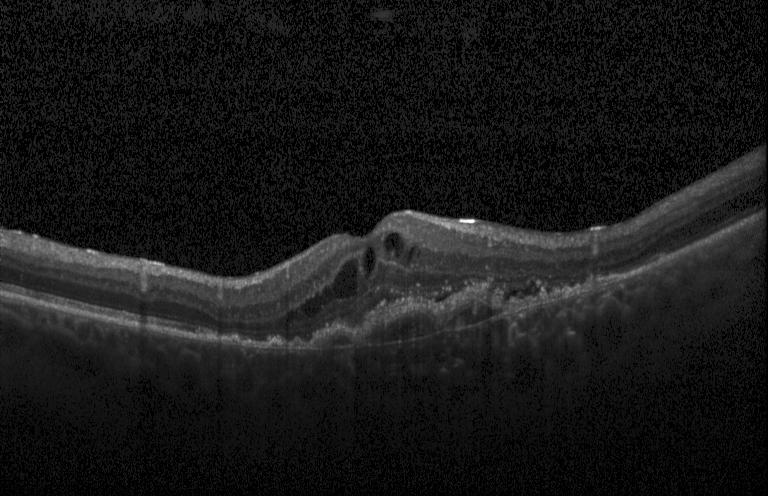

Through the macula, spectral-domain optical coherence tomography, acquired on a Heidelberg Spectralis, retinal OCT B-scan — Dx: CNV.